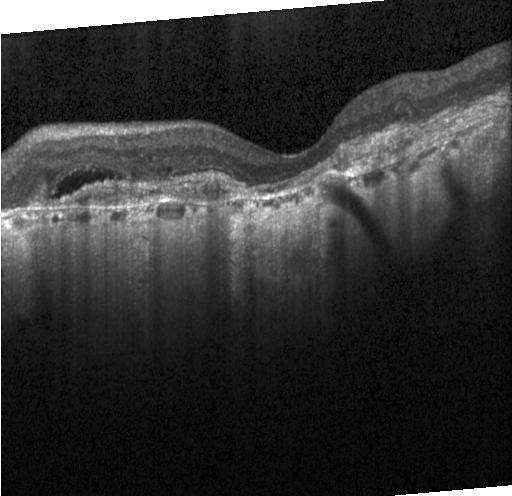
Heidelberg Spectralis OCT system; OCT line scan; spectral-domain optical coherence tomography. Dx: a choroidal neovascular membrane.